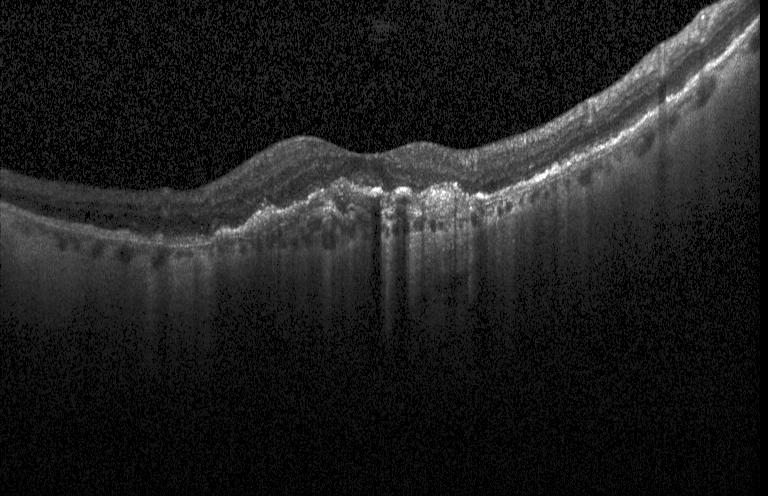
Centered on the fovea, SD-OCT, retinal OCT B-scan. Impression: a choroidal neovascular membrane.